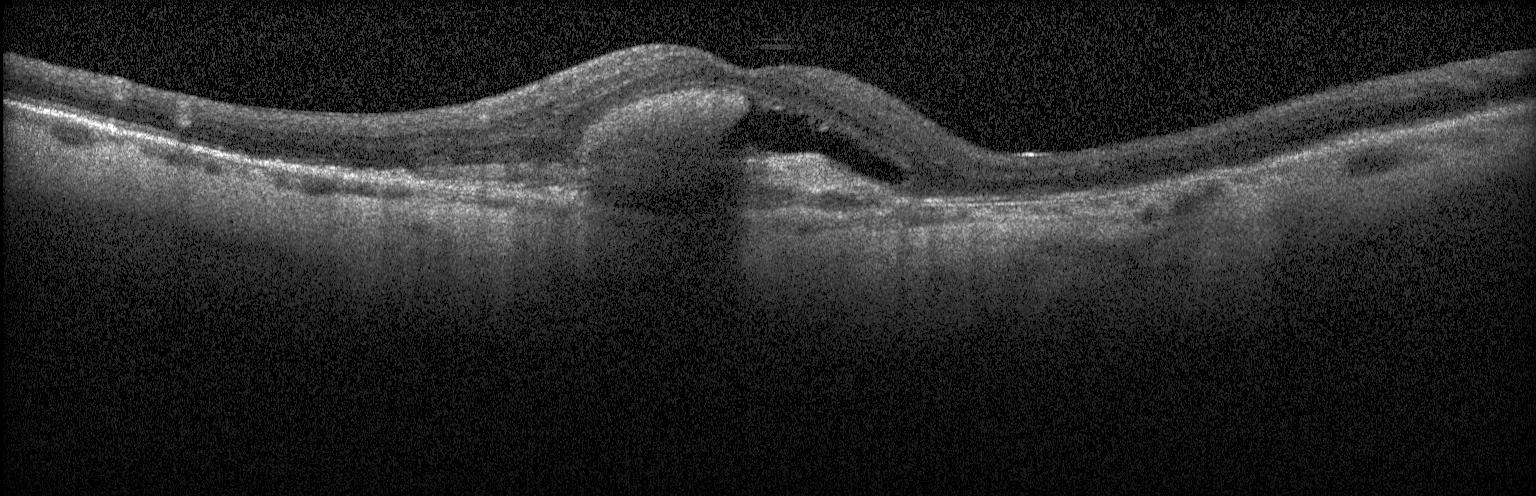 Optical coherence tomography B-scan
Finding: a choroidal neovascular membrane.